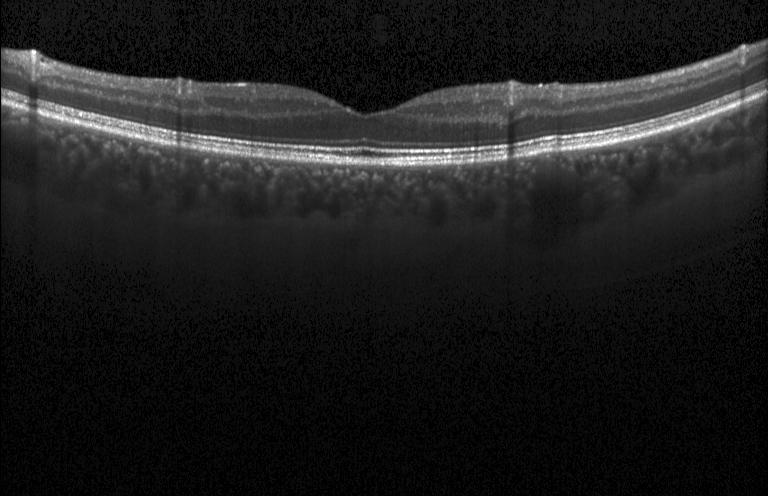
Retinal OCT B-scan, through the macula
Diagnosis: no choroidal neovascularization, diabetic macular edema, or drusen.